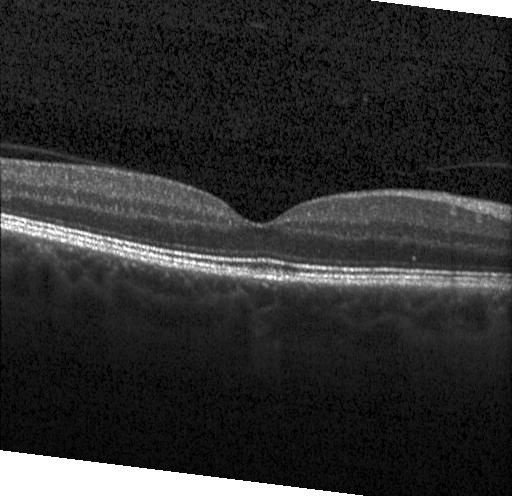
Spectral-domain optical coherence tomography · retinal OCT cross-section.
Diagnosis: no CNV, no DME, and no drusen.